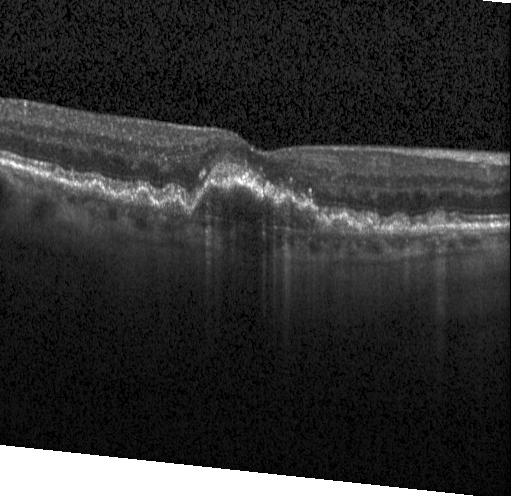 Horizontal scan through the fovea. OCT B-scan. Acquired on a Heidelberg Spectralis. SD-OCT. Diagnosis: CNV.